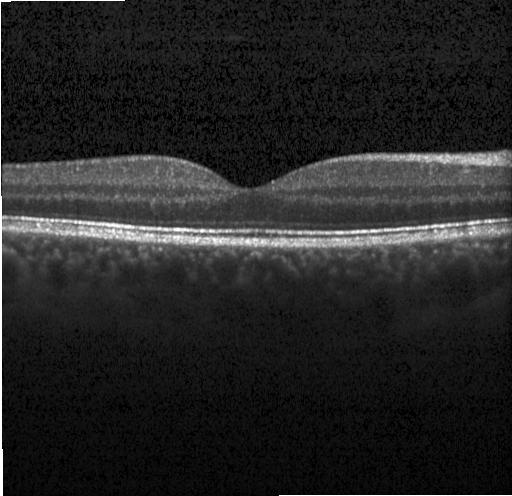

Instrument: Heidelberg Spectralis. Horizontal scan through the fovea. OCT B-scan
Macular OCT: no choroidal neovascularization, diabetic macular edema, or drusen.